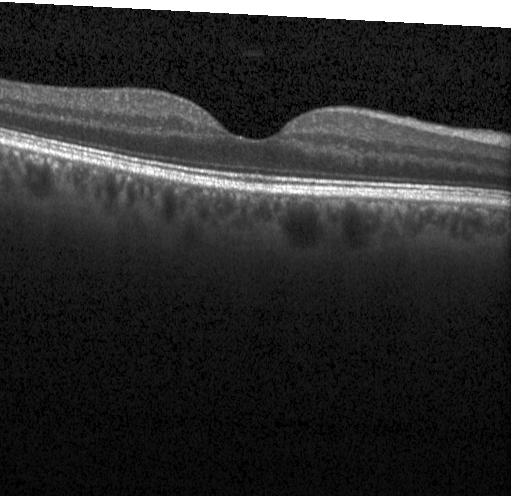 Diagnosis: no evidence of choroidal neovascularization, diabetic macular edema, or drusen.